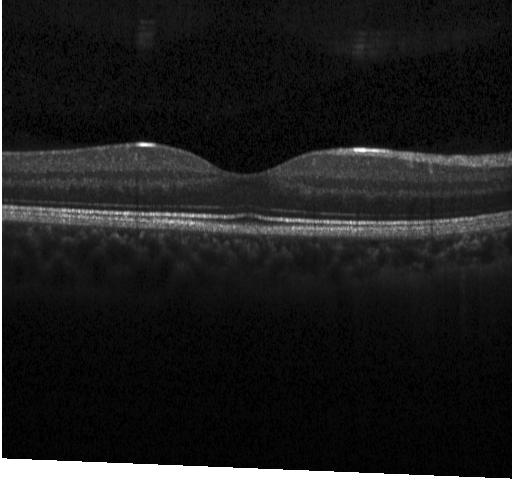
Spectral-domain OCT; optical coherence tomography B-scan.
Finding: no CNV, no DME, and no drusen.